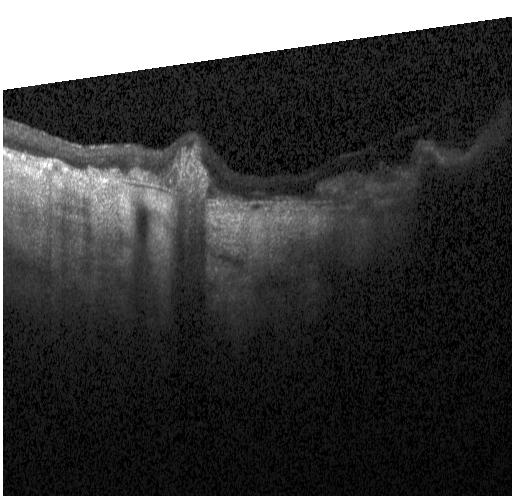
Dx: a choroidal neovascular membrane.